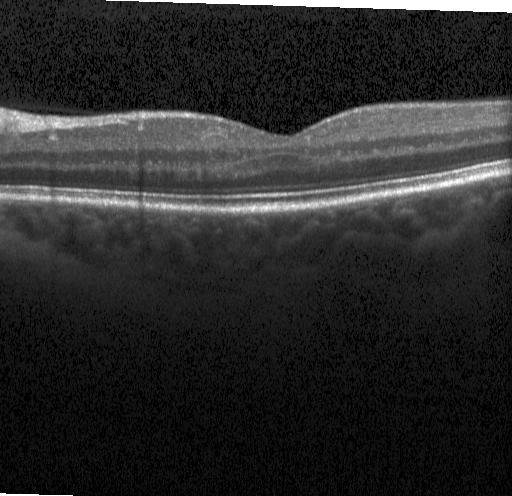

Centered on the fovea. OCT B-scan. SD-OCT.
The scan shows no evidence of choroidal neovascularization, diabetic macular edema, or drusen.